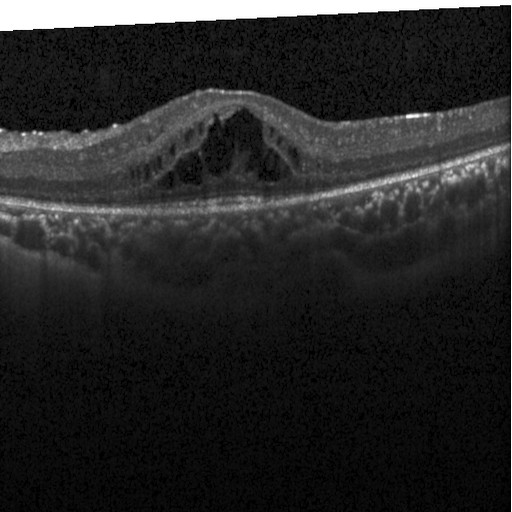
Finding: diabetic macular edema (DME).